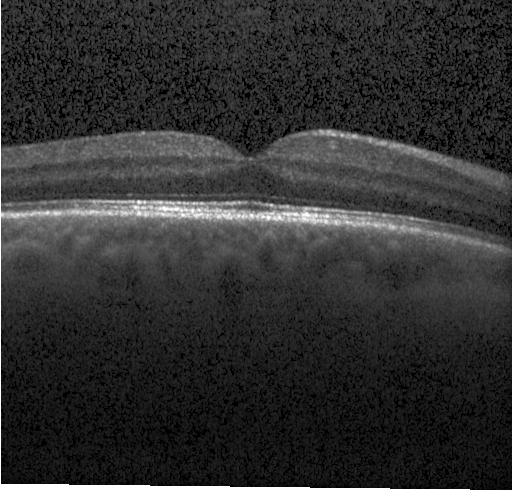 Optical coherence tomography scan · SD-OCT.
This B-scan demonstrates no evidence of choroidal neovascularization, diabetic macular edema, or drusen.